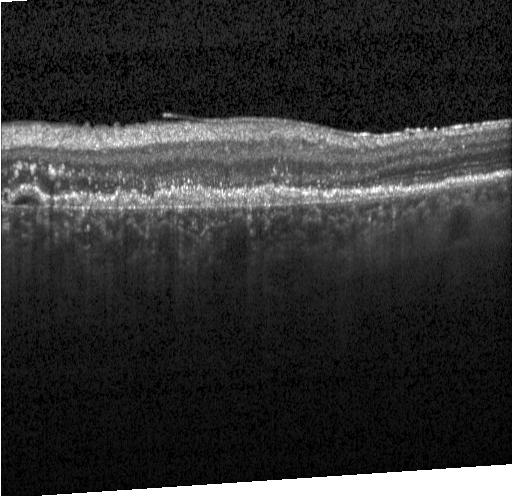

CNV.